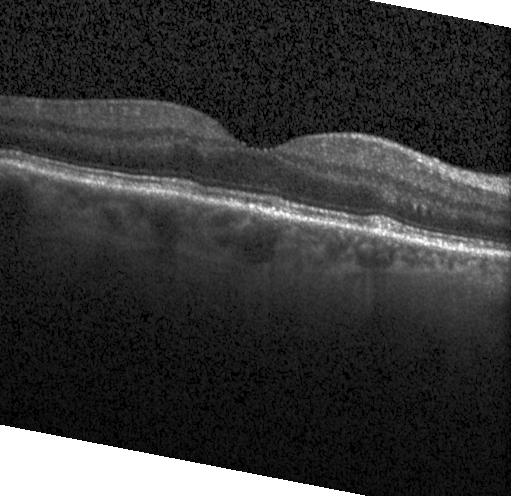

Spectral-domain OCT, OCT B-scan, fovea-centered. Impression: no choroidal neovascularization, no diabetic macular edema, and no drusen.